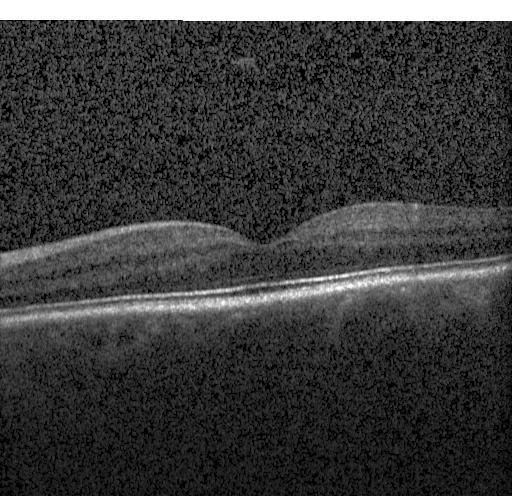

Spectral-domain OCT B-scan: no evidence of CNV, DME, or drusen.